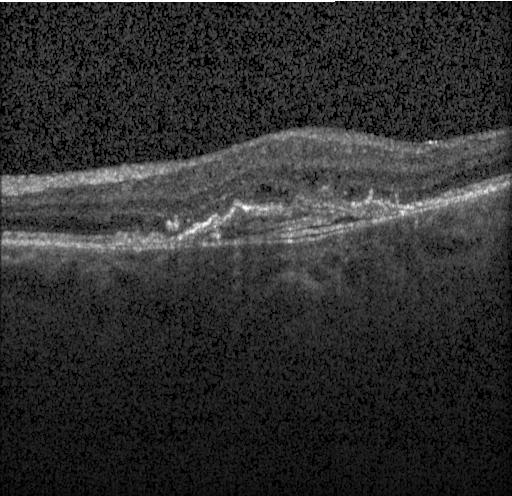

Fovea-centered, spectral-domain OCT, retinal OCT B-scan. Diagnosis: a choroidal neovascular membrane.